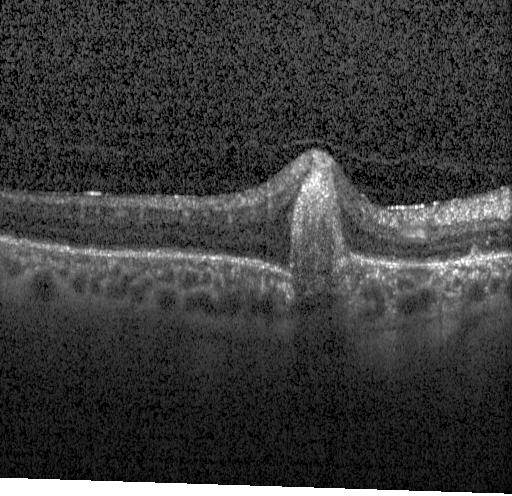
OCT line scan, fovea-centered
Diagnosis: a choroidal neovascular membrane.